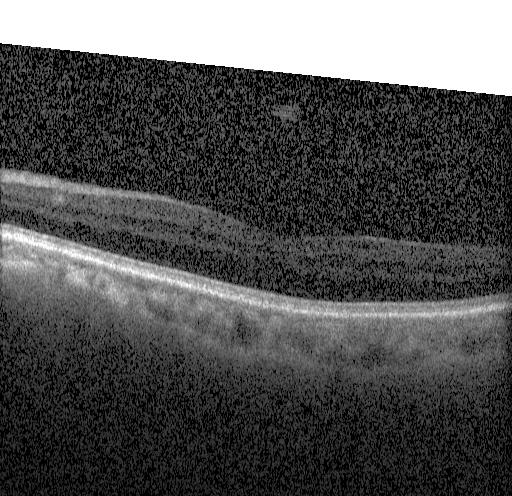 Impression: no evidence of choroidal neovascularization, diabetic macular edema, or drusen.